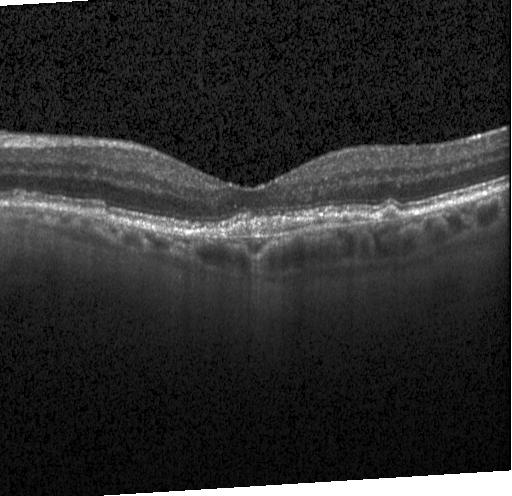
Spectral-domain OCT B-scan: a choroidal neovascular membrane.